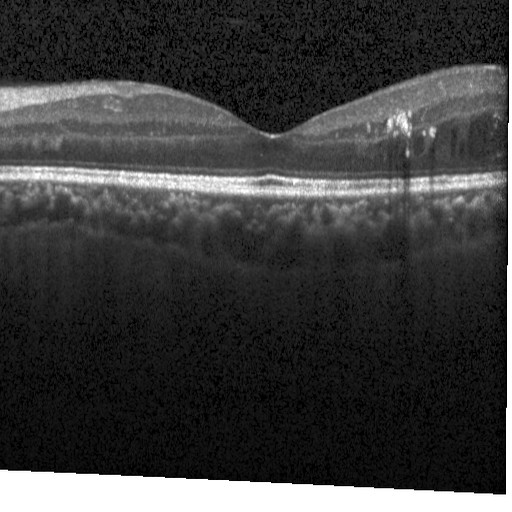

Finding: diabetic macular edema (DME).